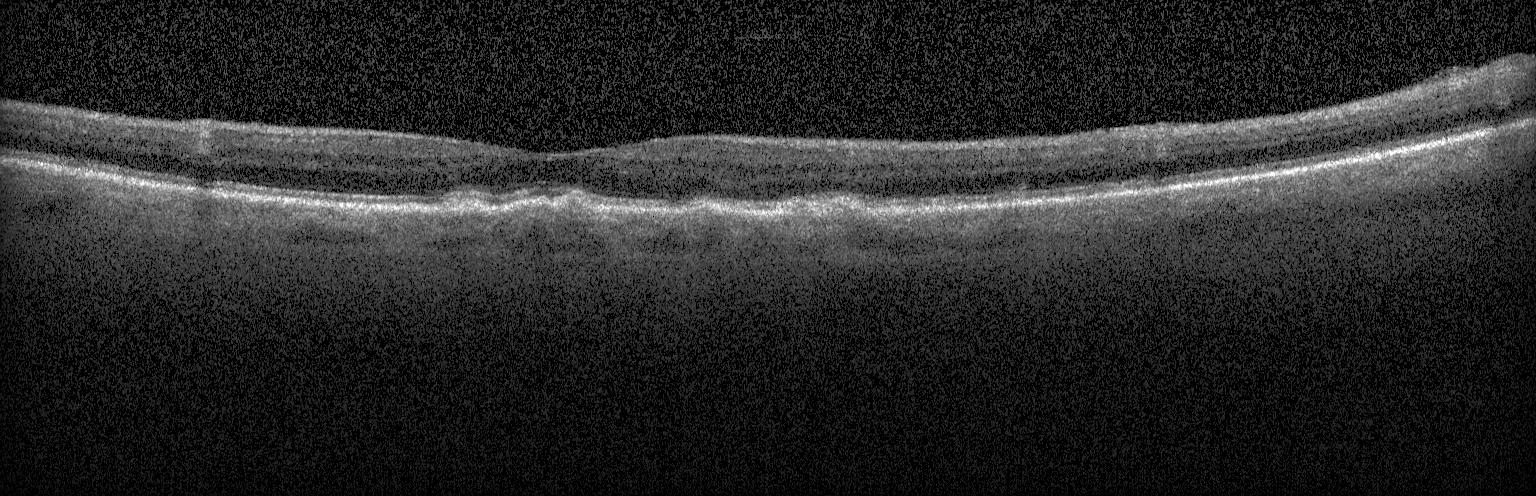

OCT B-scan. Spectral-domain optical coherence tomography. Instrument: Heidelberg Spectralis. Fovea-centered. Impression: sub-RPE drusenoid deposits.